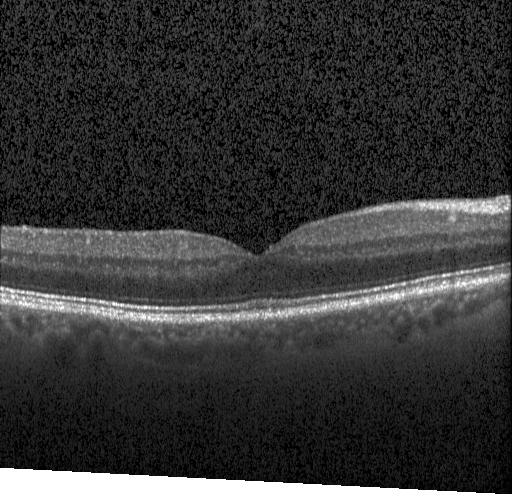
Through the macula, acquired on a Heidelberg Spectralis, spectral-domain OCT, retinal OCT B-scan. Dx: neither CNV, DME, nor drusen.